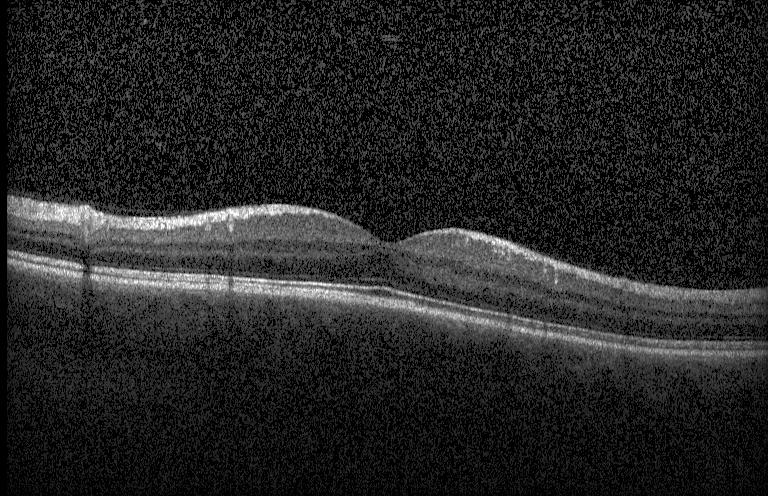 Impression: no choroidal neovascularization, no diabetic macular edema, and no drusen.